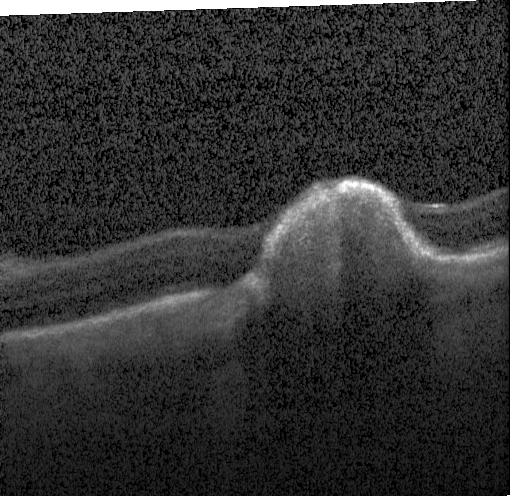
Macular OCT: choroidal neovascularization (CNV).